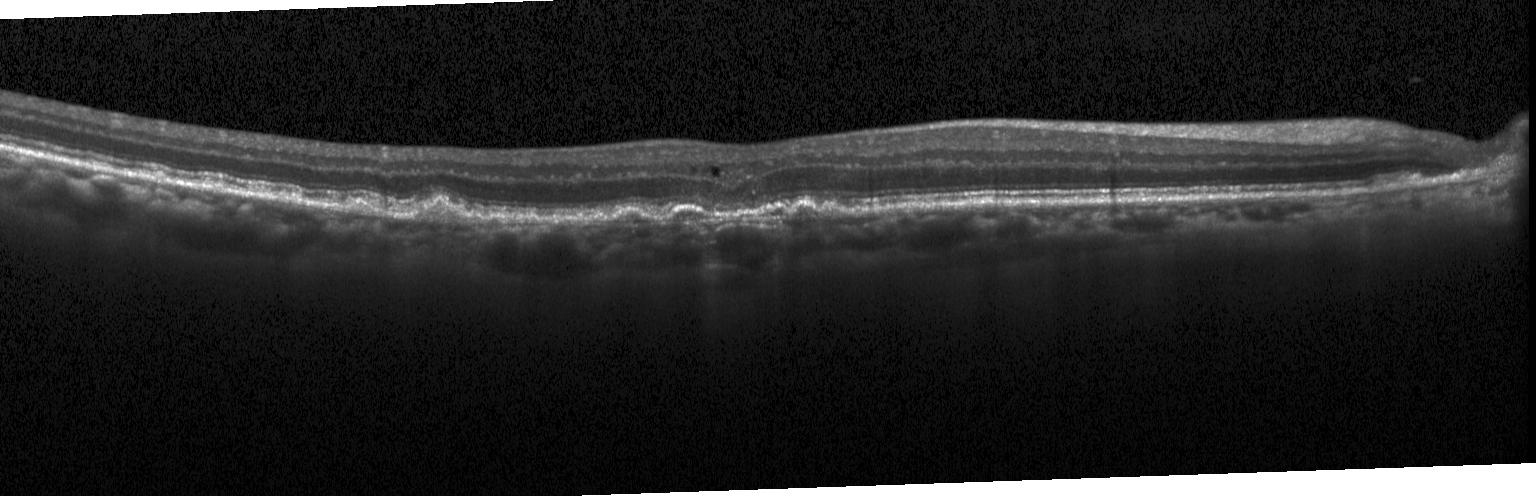

OCT B-scan showing choroidal neovascularization (CNV).